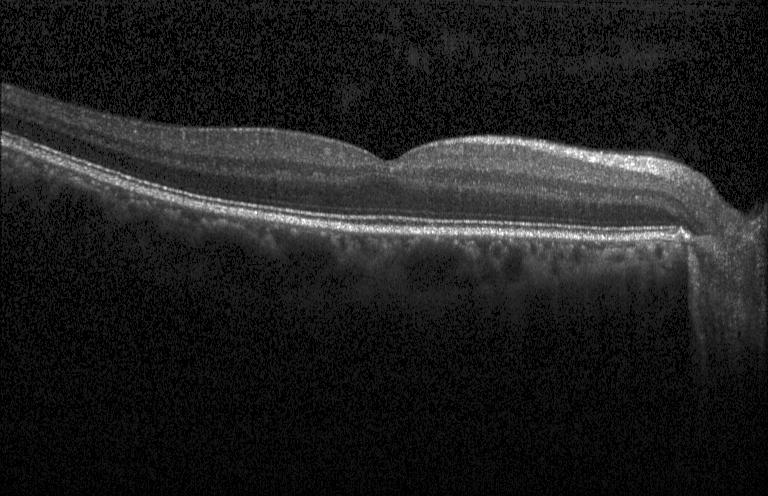 Retinal OCT cross-section showing neither CNV, DME, nor drusen.